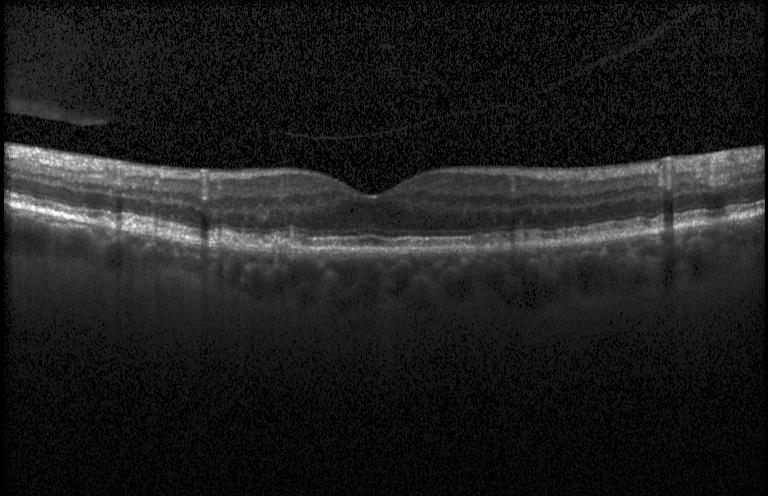

Retinal OCT cross-section — Finding: drusen.